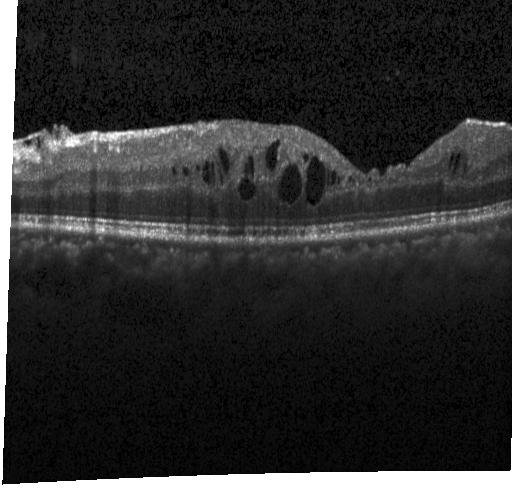 OCT line scan — Macular OCT: diabetic macular edema.